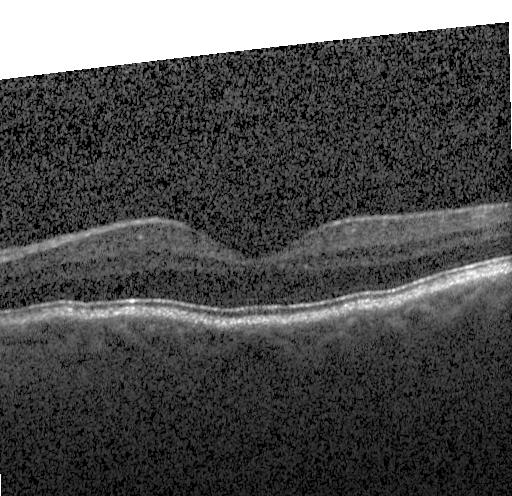
Optical coherence tomography scan.
Impression: no choroidal neovascularization, diabetic macular edema, or drusen.